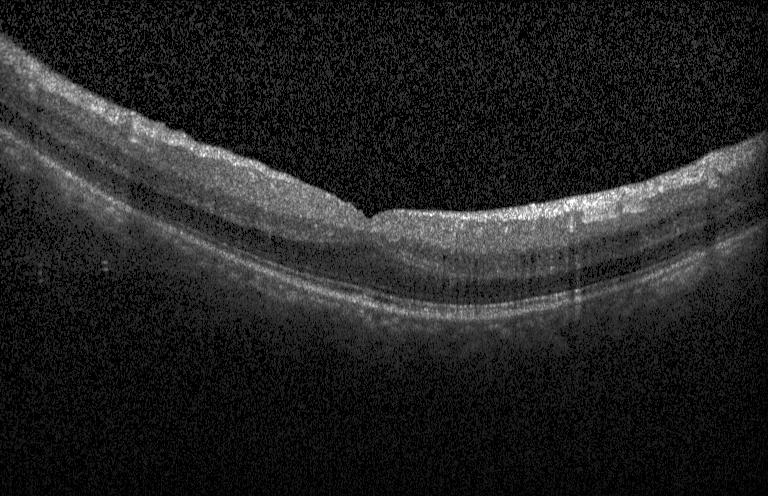
This B-scan demonstrates diabetic macular edema.